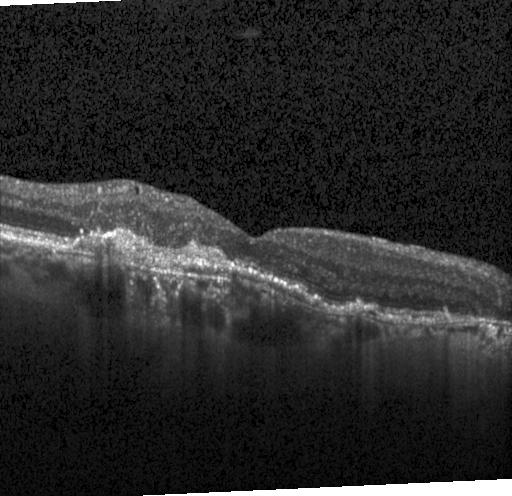
Retinal OCT cross-section.
Assessment: choroidal neovascularization (CNV).